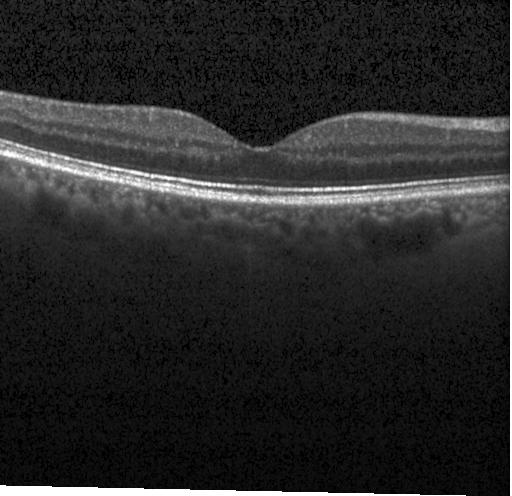
Macular OCT: neither CNV, DME, nor drusen.